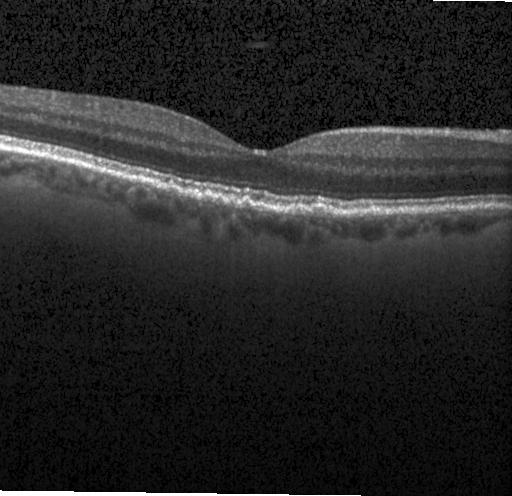
OCT finding: sub-RPE drusenoid deposits.